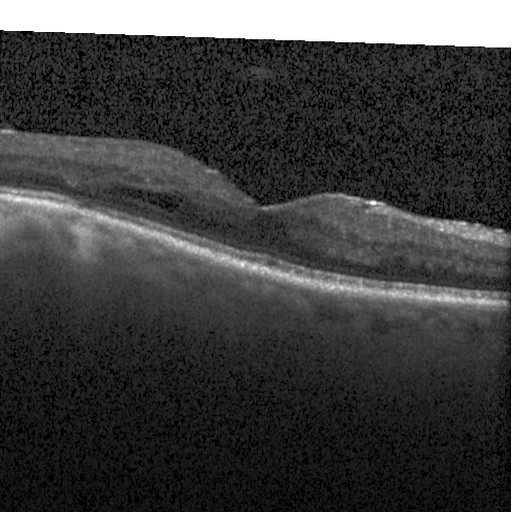
Retinal OCT B-scan.
Finding: DME.